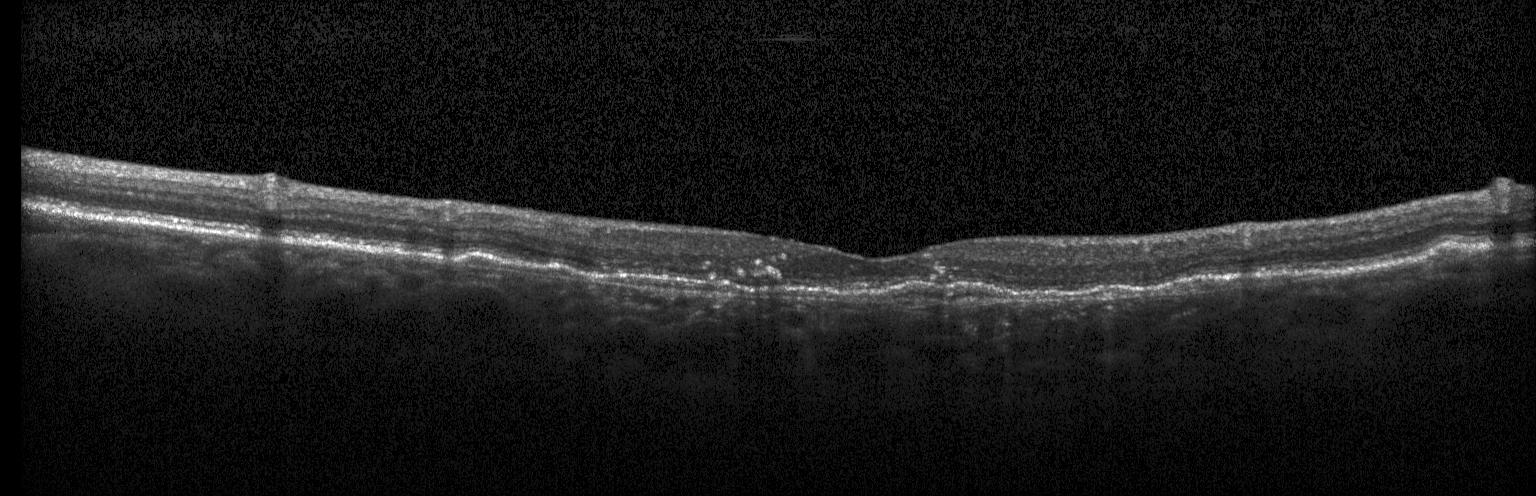

Dx: a choroidal neovascular membrane.